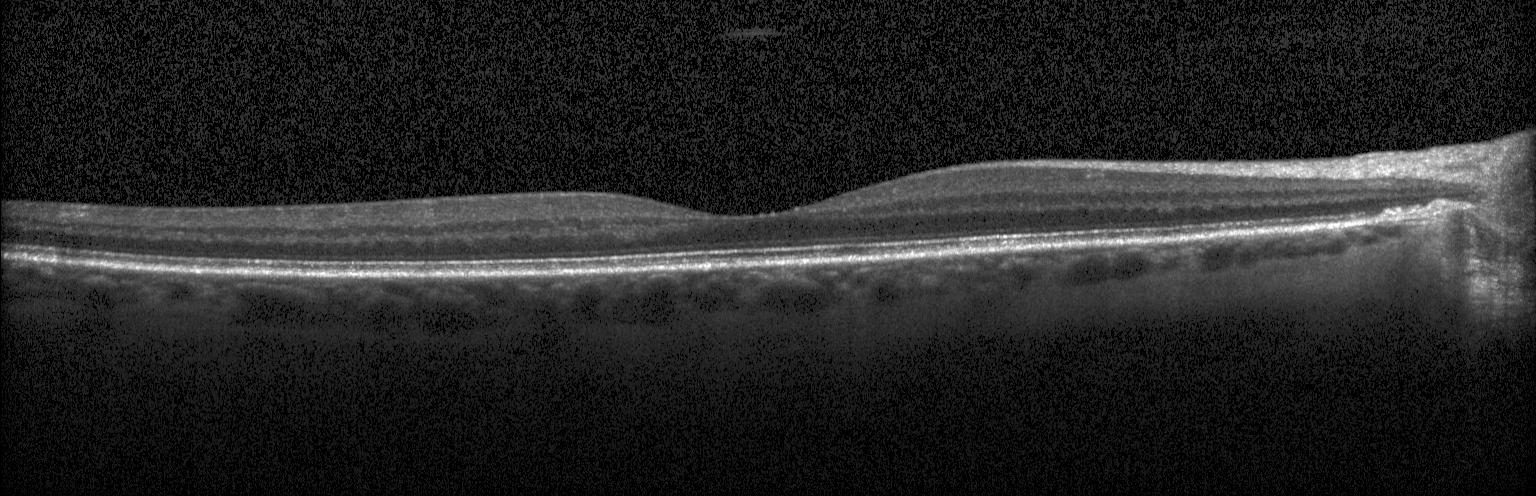
OCT line scan; spectral-domain optical coherence tomography; through the macula; acquired on a Heidelberg Spectralis.
Impression: neither choroidal neovascularization, diabetic macular edema, nor drusen.